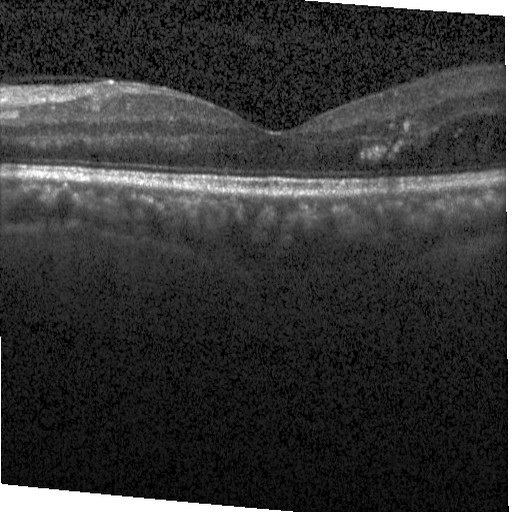

SD-OCT. Optical coherence tomography B-scan. Horizontal scan through the fovea. Heidelberg Spectralis OCT system — Impression: diabetic macular edema.